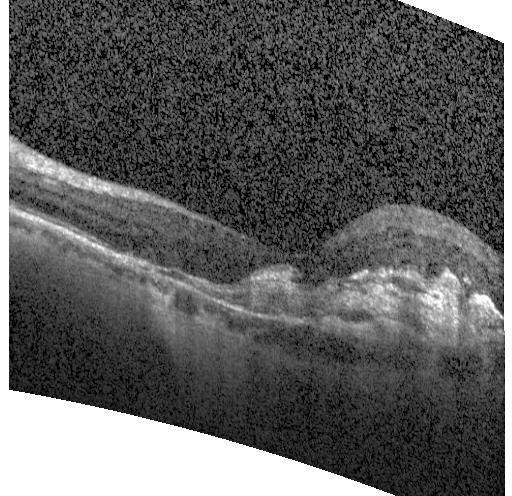
Retinal OCT B-scan. Horizontal scan through the fovea. Heidelberg Spectralis OCT system — Finding: a choroidal neovascular membrane.